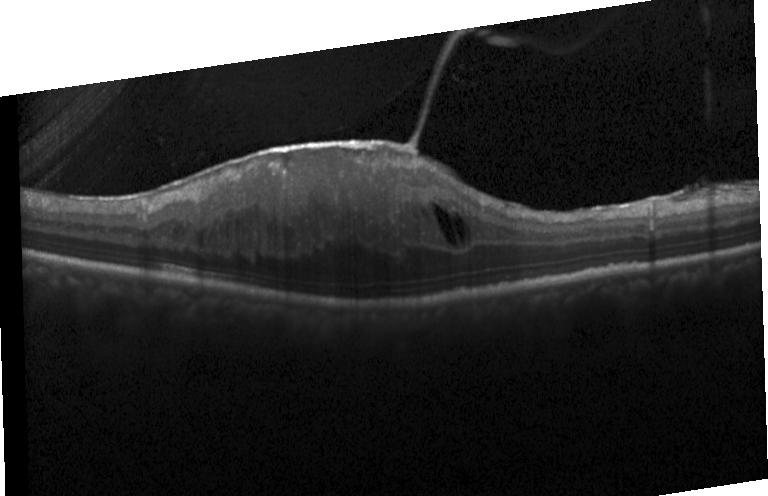
Finding: diabetic macular edema.